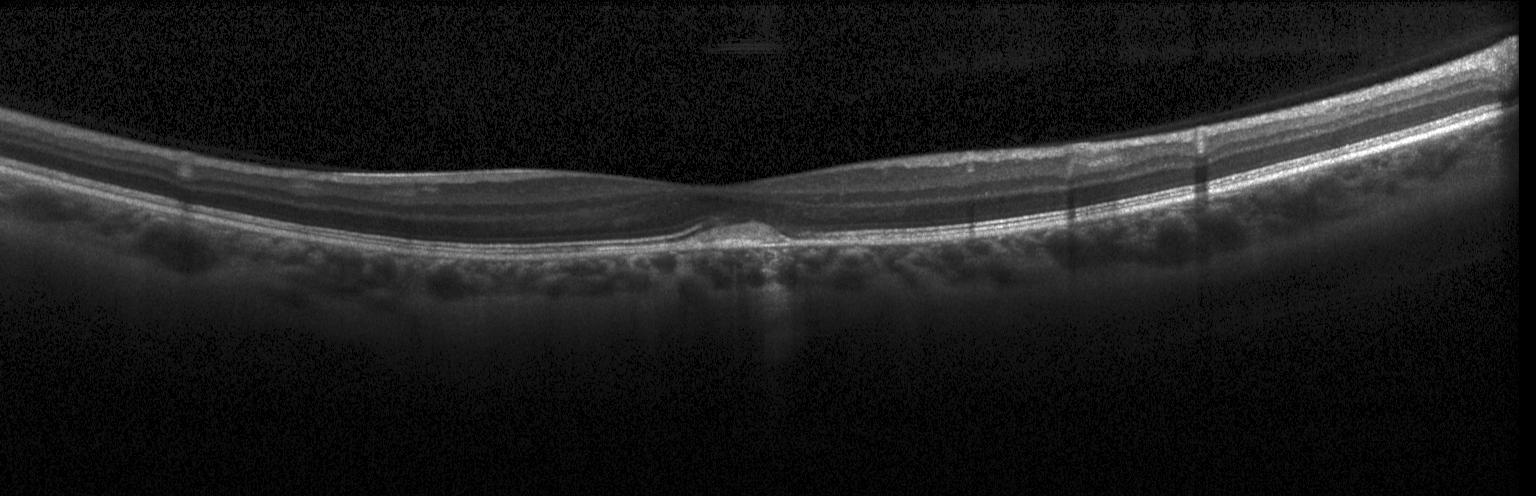

Retinal OCT cross-section
This B-scan demonstrates choroidal neovascularization.